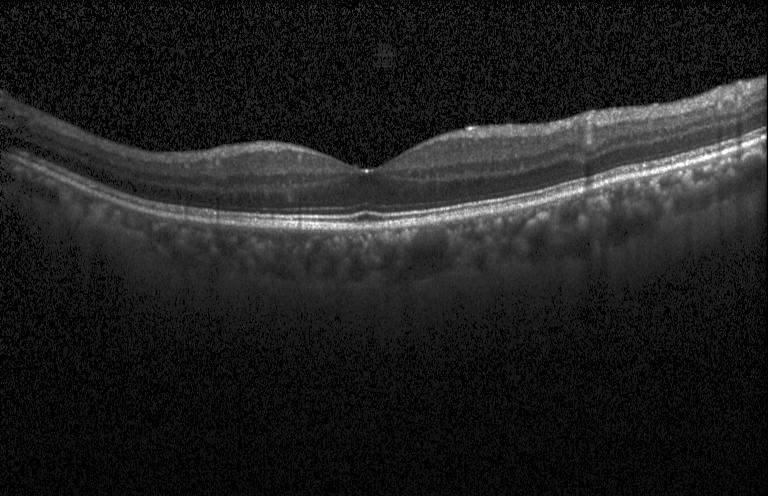

OCT scan showing no CNV, DME, or drusen.